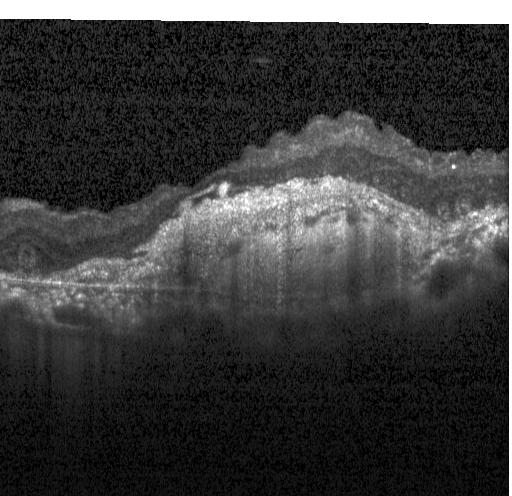 OCT finding: a choroidal neovascular membrane.